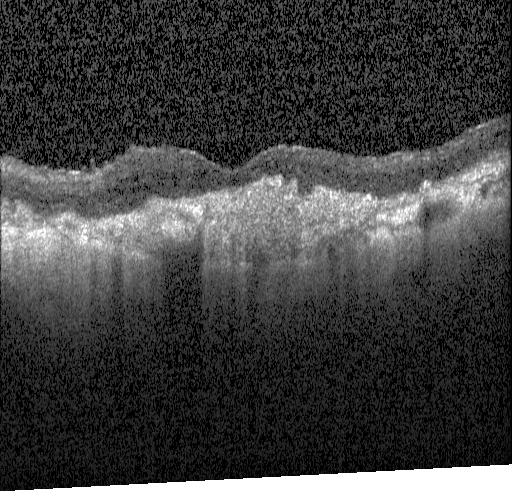 Retinal OCT cross-section; centered on the fovea; spectral-domain optical coherence tomography.
Finding: a choroidal neovascular membrane.